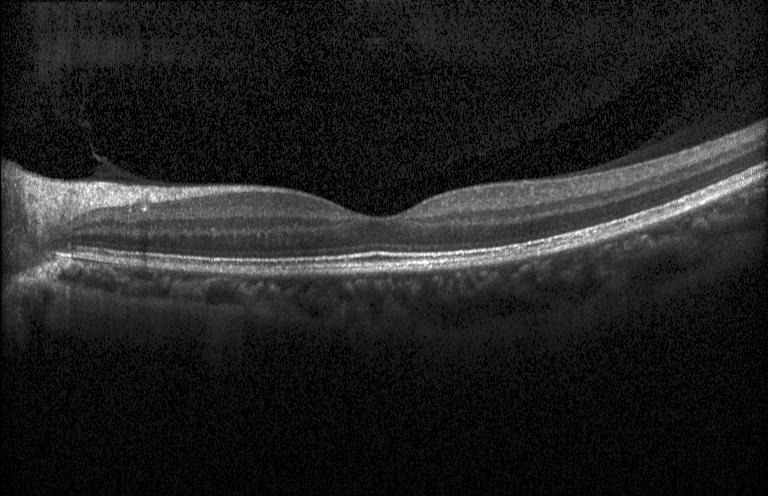 Retinal OCT cross-section showing no evidence of choroidal neovascularization, diabetic macular edema, or drusen.